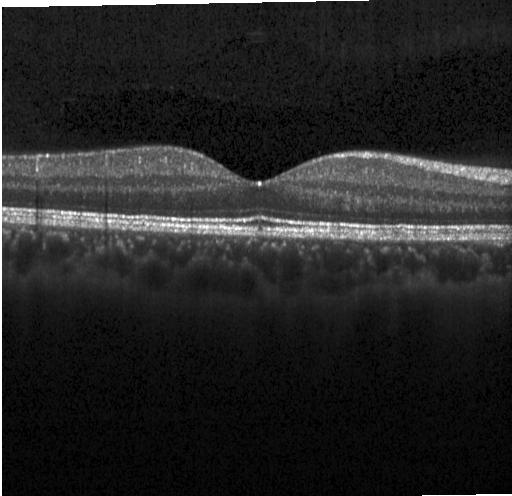 Retinal OCT cross-section. Diagnosis: no choroidal neovascularization, no diabetic macular edema, and no drusen.